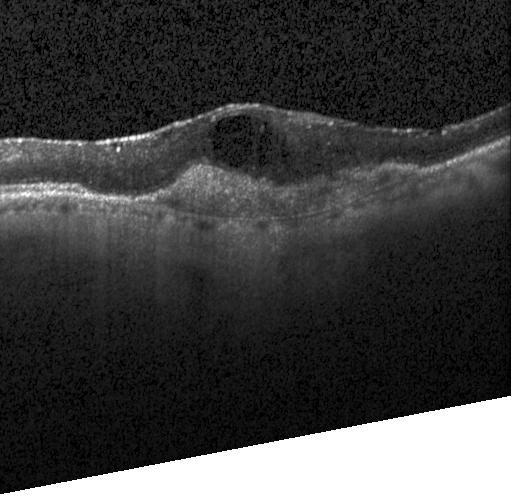
Heidelberg Spectralis. Retinal OCT B-scan.
Impression: CNV.